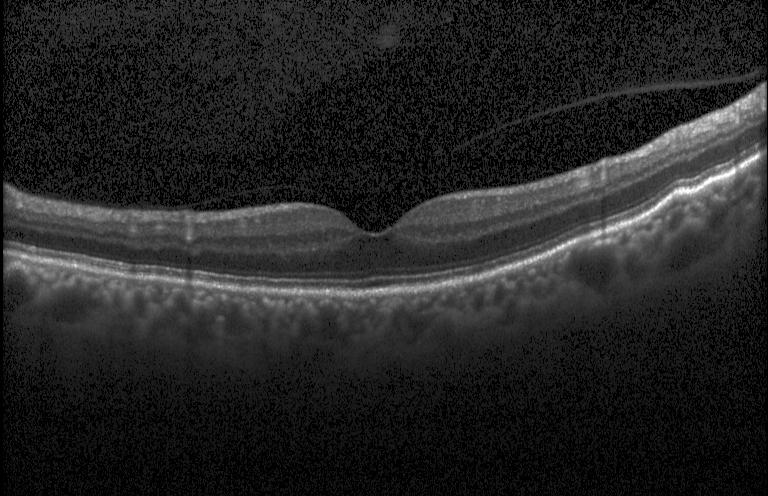

Spectral-domain OCT · retinal OCT B-scan · Heidelberg Spectralis OCT system · horizontal scan through the fovea
Impression: neither choroidal neovascularization, diabetic macular edema, nor drusen.